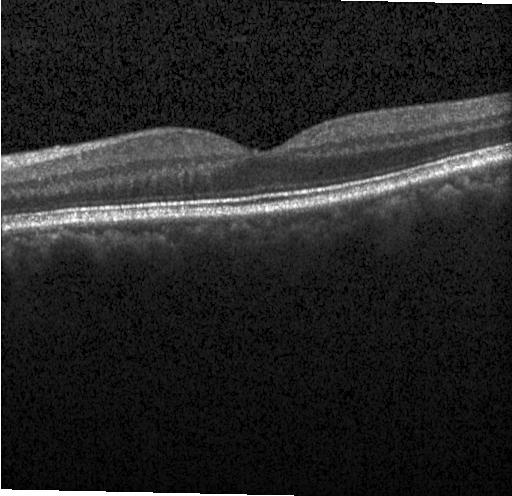

OCT B-scan; Heidelberg Spectralis. Dx: neither CNV, DME, nor drusen.